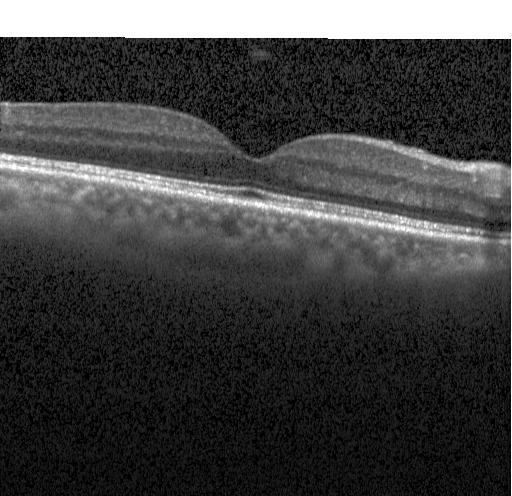
Diagnosis: neither CNV, DME, nor drusen.